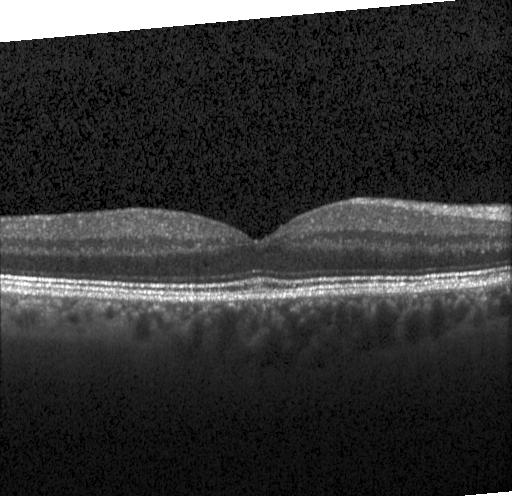

The scan shows no CNV, DME, or drusen.